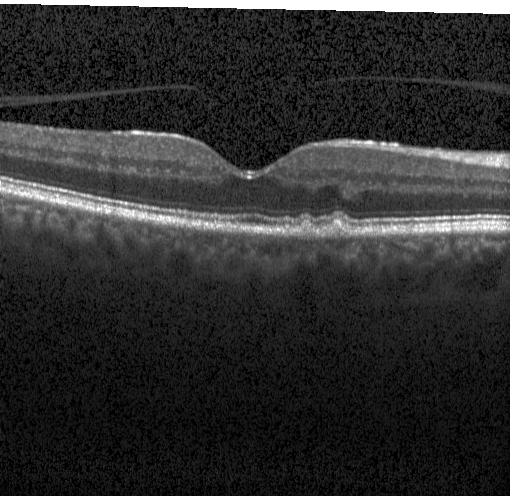 OCT scan showing sub-RPE drusenoid deposits.